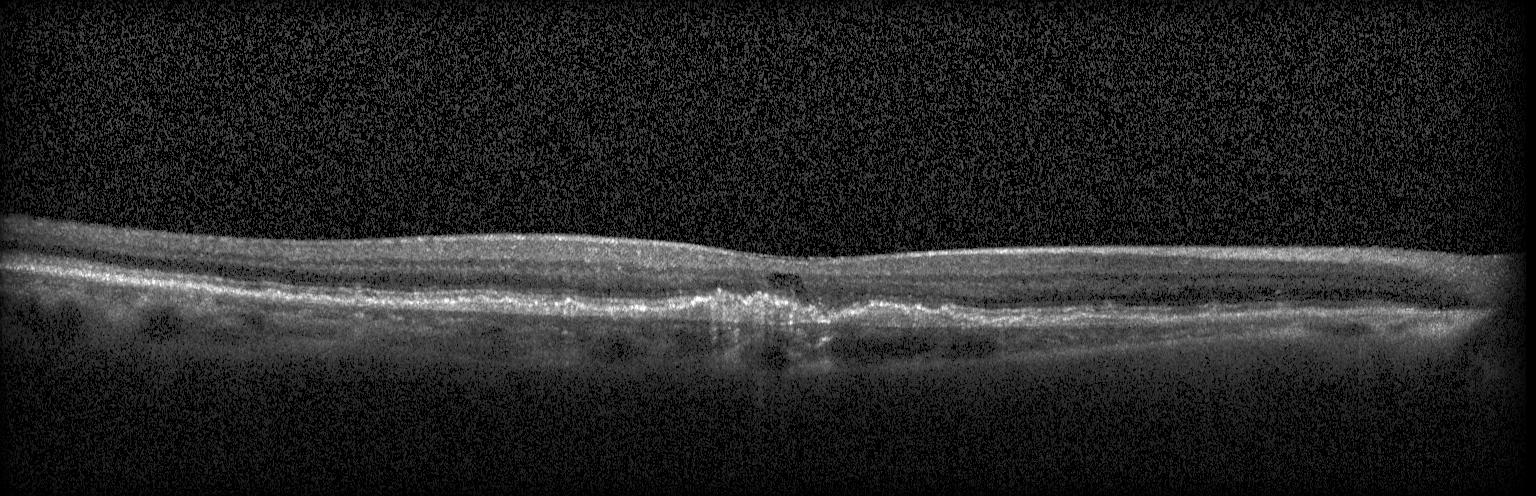

Optical coherence tomography B-scan.
Choroidal neovascularization (CNV).